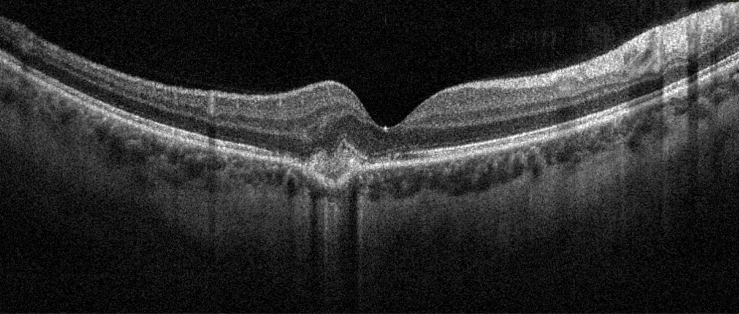 OCT scan showing age-related macular degeneration (AMD).